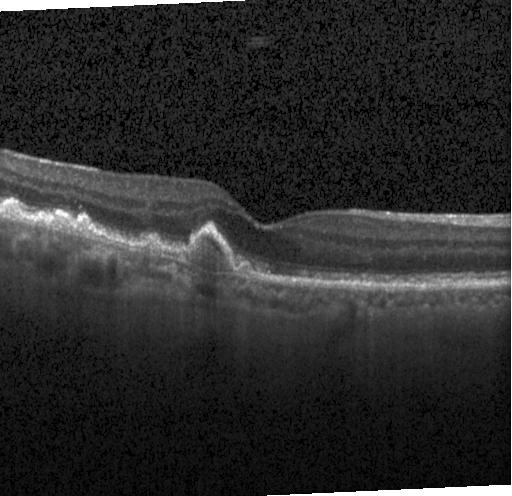

Through the macula. Heidelberg Spectralis. Spectral-domain optical coherence tomography. Retinal OCT cross-section — Impression: drusen.